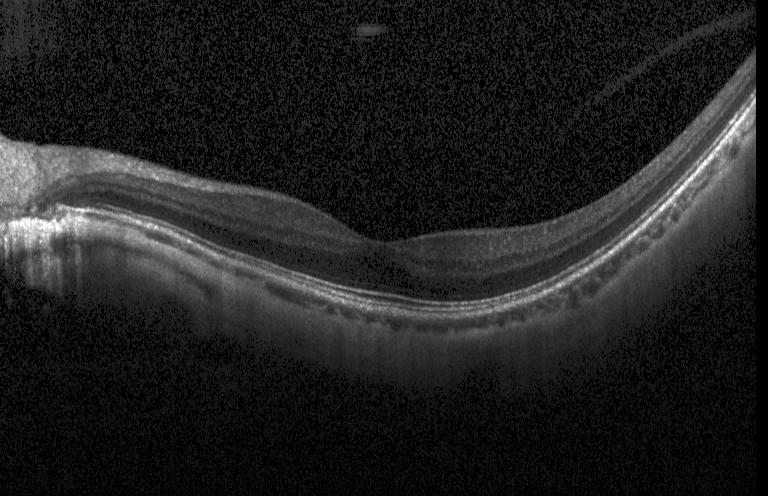 Centered on the fovea; instrument: Heidelberg Spectralis; optical coherence tomography scan
Finding: no CNV, no DME, and no drusen.